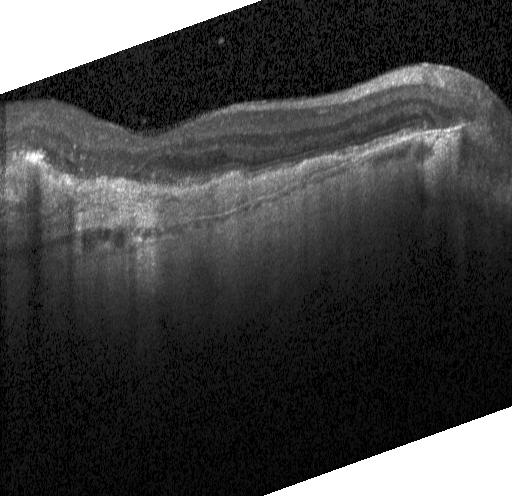

Heidelberg Spectralis OCT system. Retinal OCT B-scan
Impression: CNV.